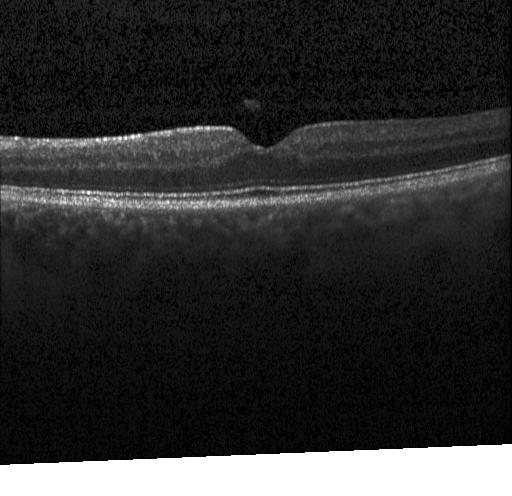 Impression: no choroidal neovascularization, diabetic macular edema, or drusen.